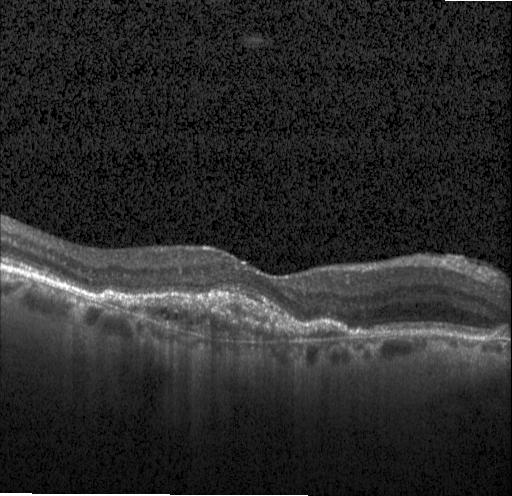 Optical coherence tomography B-scan. Centered on the fovea. Heidelberg Spectralis
This B-scan demonstrates a choroidal neovascular membrane.